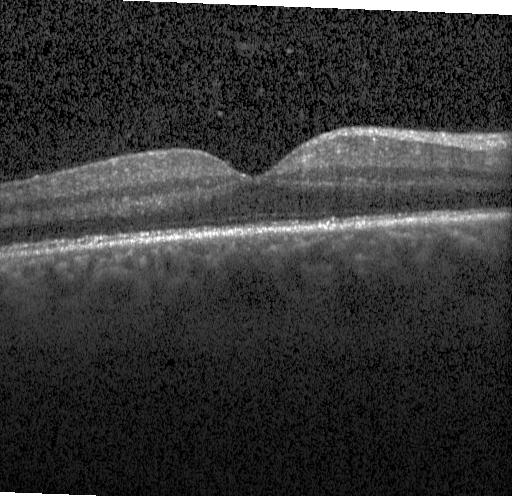

Macular OCT demonstrating no choroidal neovascularization, no diabetic macular edema, and no drusen.